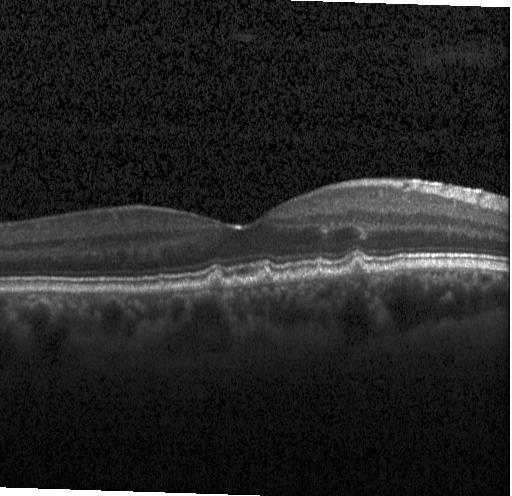 OCT B-scan showing multiple drusen.